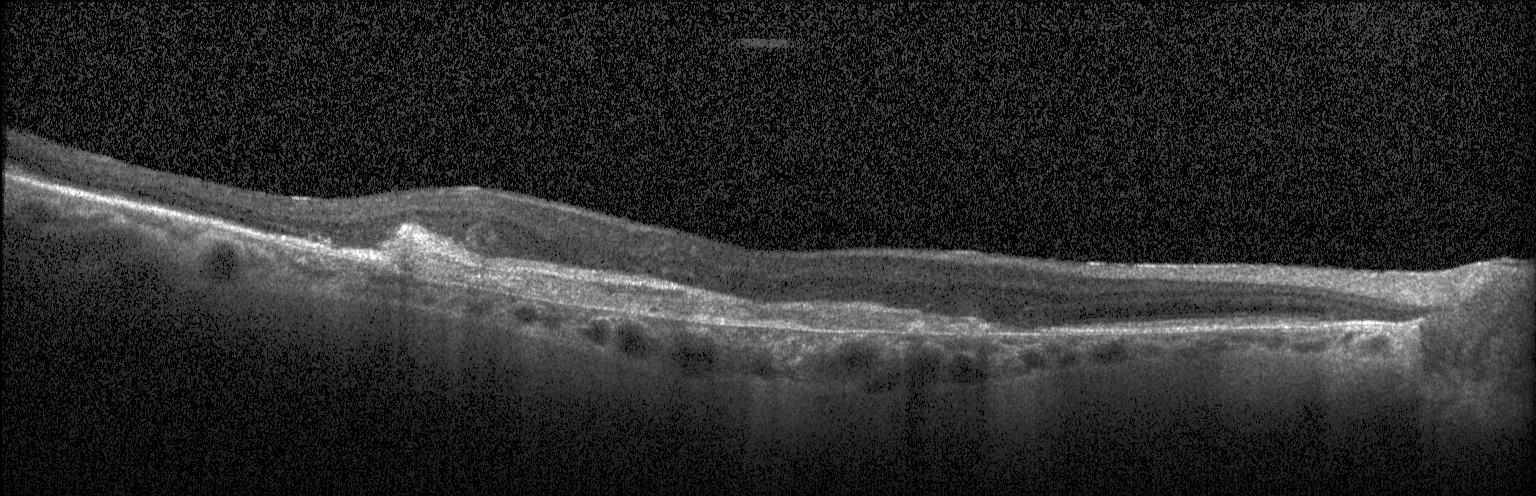

Macular OCT demonstrating choroidal neovascularization (CNV).